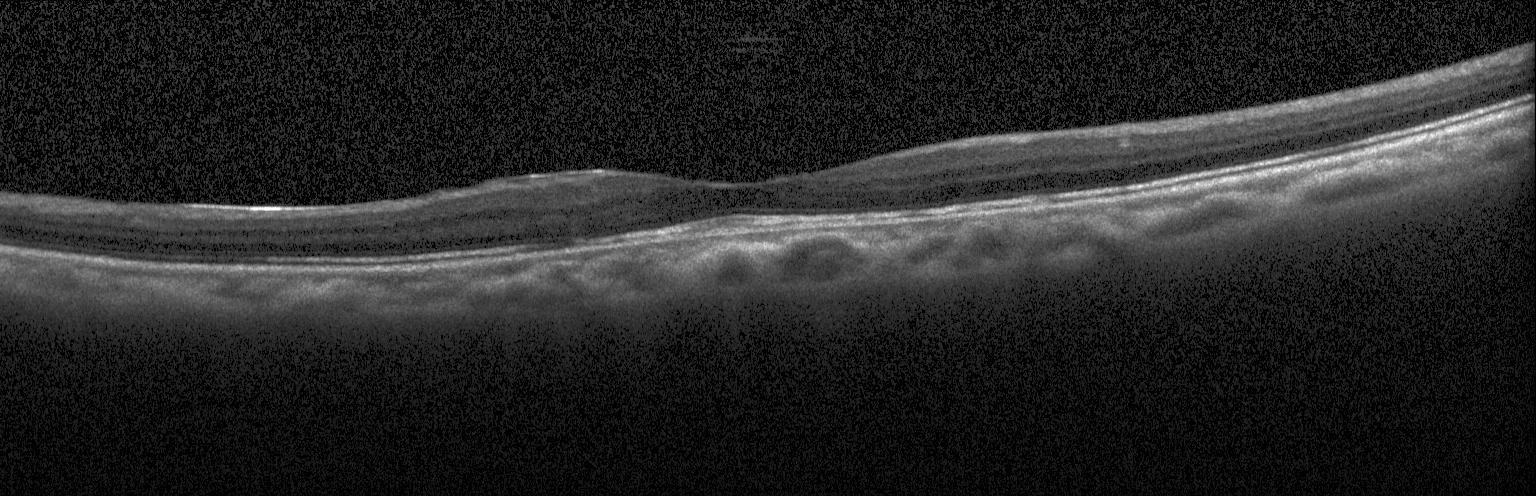

OCT B-scan, instrument: Heidelberg Spectralis, fovea-centered, spectral-domain optical coherence tomography — Impression: neither CNV, DME, nor drusen.